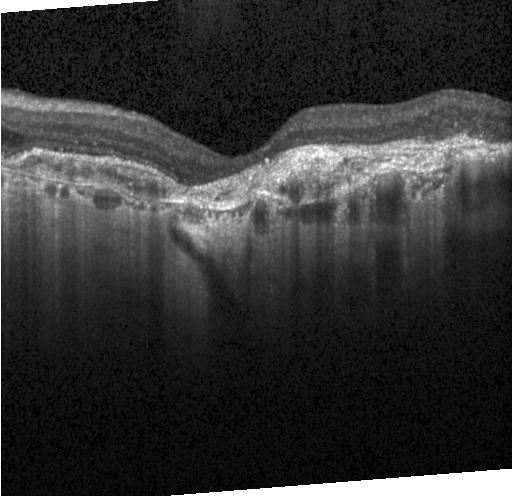
Fovea-centered, retinal OCT cross-section, instrument: Heidelberg Spectralis, spectral-domain optical coherence tomography
Macular OCT: choroidal neovascularization.